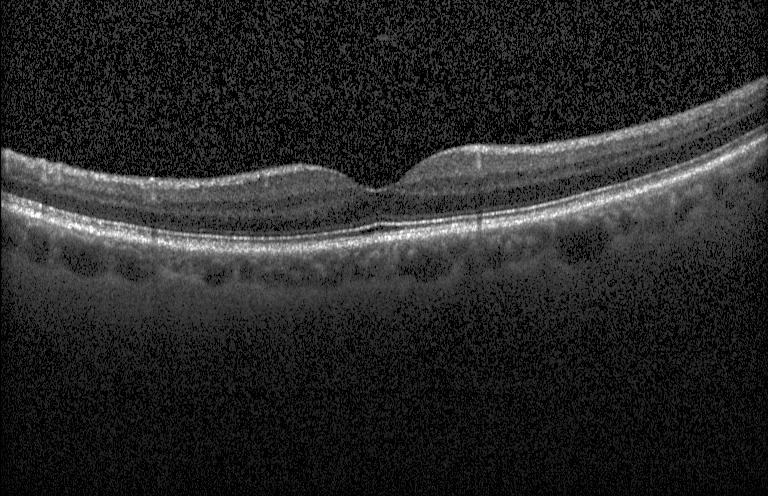

Retinal OCT cross-section
Impression: no CNV, DME, or drusen.